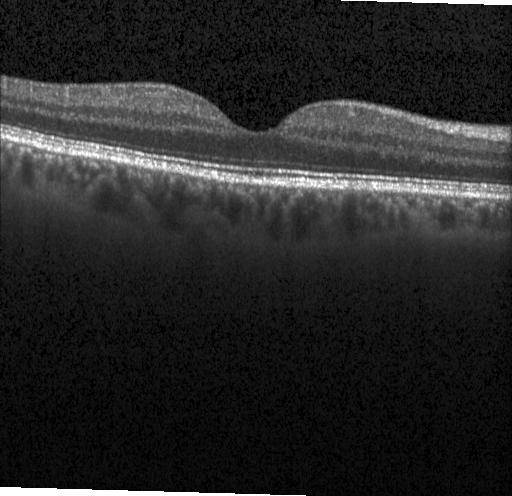 OCT B-scan, spectral-domain OCT, Heidelberg Spectralis OCT system
Impression: no evidence of choroidal neovascularization, diabetic macular edema, or drusen.